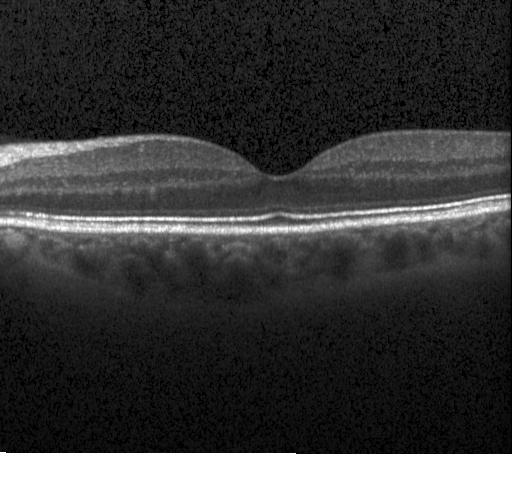
Horizontal scan through the fovea; retinal OCT B-scan; Heidelberg Spectralis OCT system
Impression: no choroidal neovascularization, diabetic macular edema, or drusen.